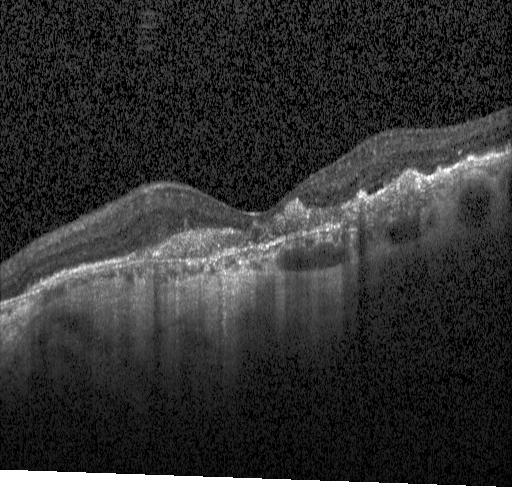 Macular OCT demonstrating a choroidal neovascular membrane.